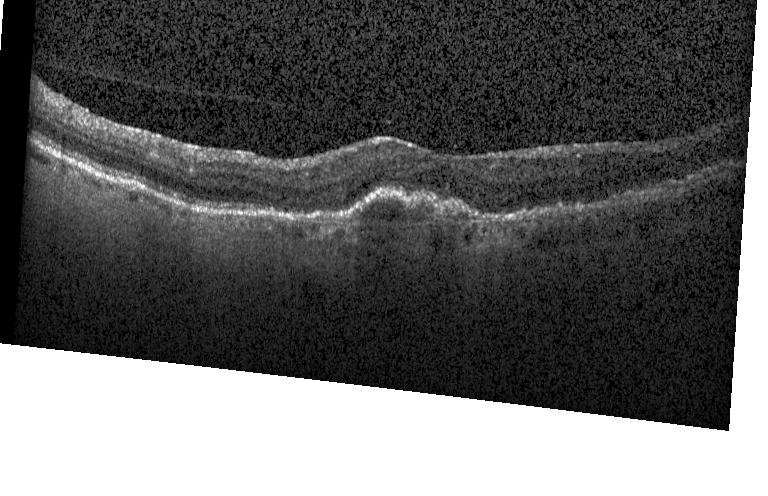
Macular OCT: a choroidal neovascular membrane.